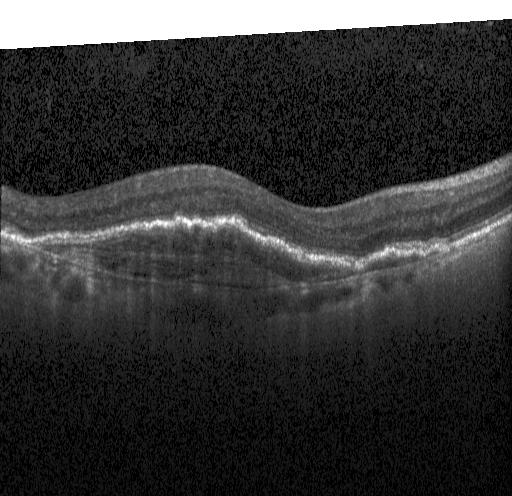

Optical coherence tomography B-scan, acquired on a Heidelberg Spectralis, macular scan — Impression: a choroidal neovascular membrane.